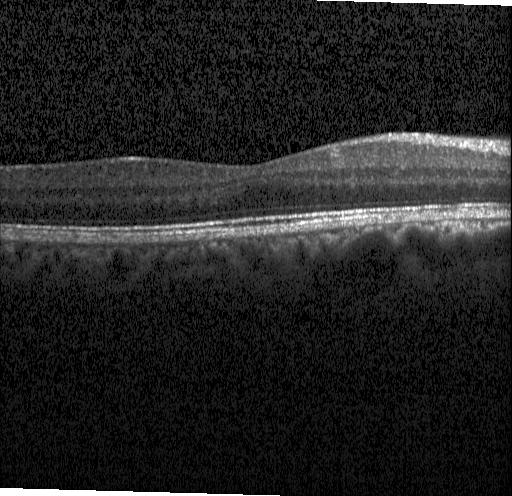 Optical coherence tomography B-scan. Horizontal scan through the fovea. SD-OCT. Finding: neither CNV, DME, nor drusen.